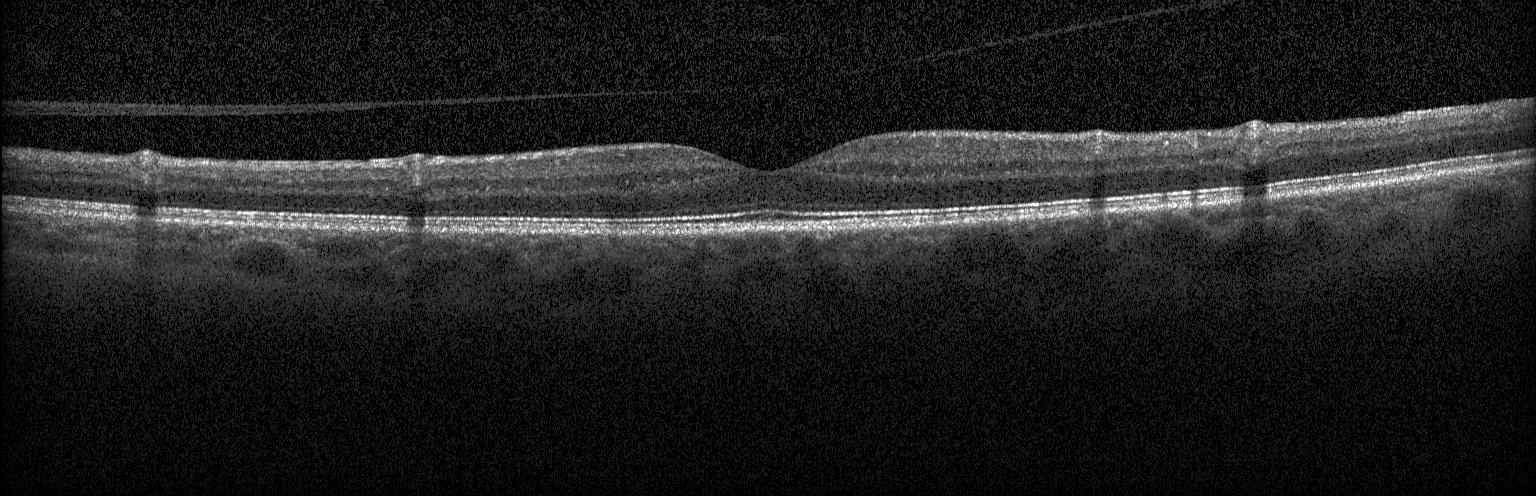
OCT finding: no CNV, DME, or drusen.